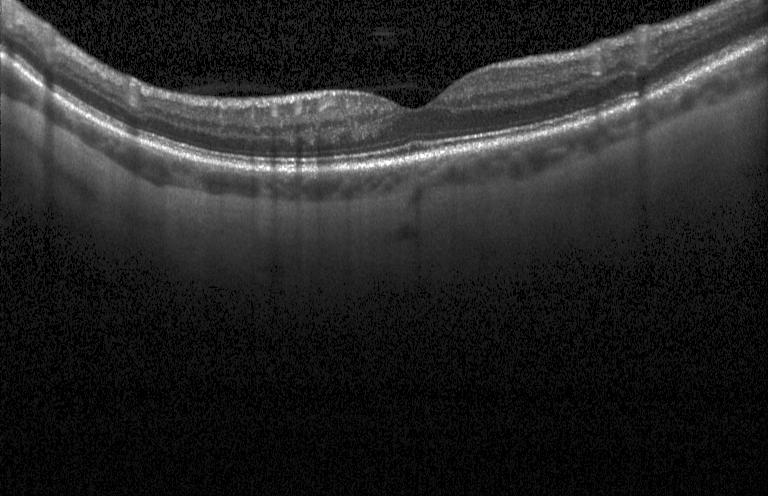

Retinal OCT cross-section, SD-OCT
Impression: no choroidal neovascularization, no diabetic macular edema, and no drusen.